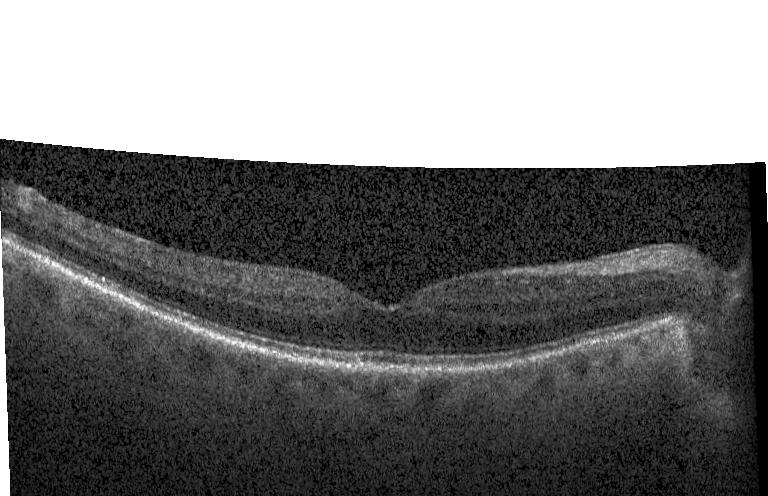 Spectral-domain OCT · horizontal scan through the fovea · OCT B-scan
No evidence of choroidal neovascularization, diabetic macular edema, or drusen.